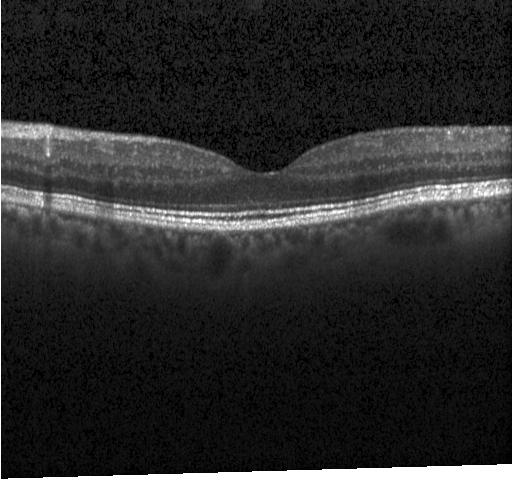

No choroidal neovascularization, no diabetic macular edema, and no drusen.